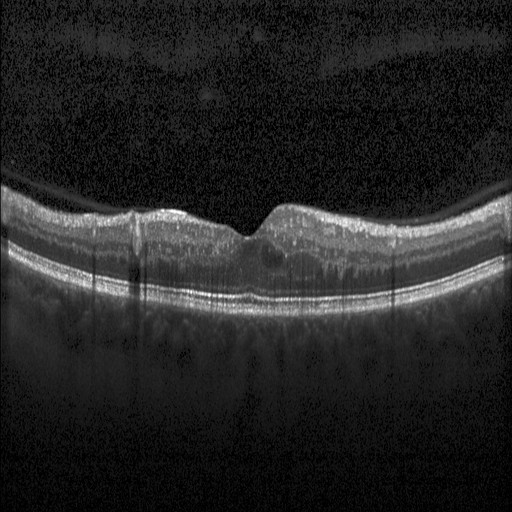
Retinal OCT B-scan. The scan shows diabetic macular edema.